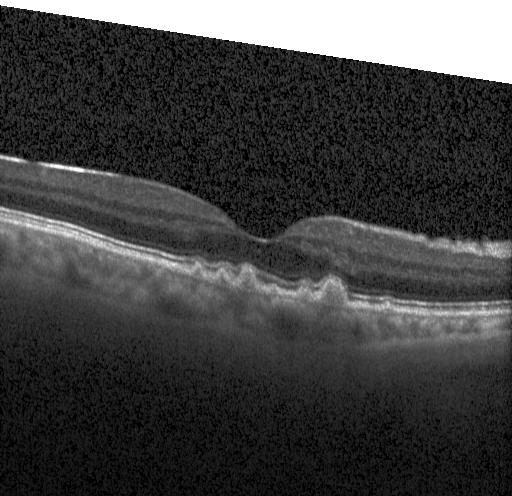
Retinal OCT B-scan — Impression: drusen.